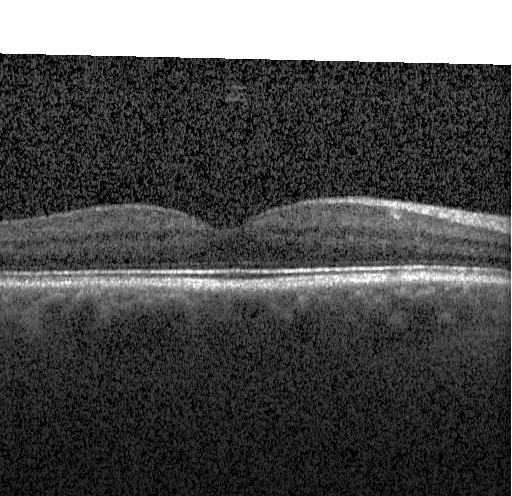 Impression: no evidence of choroidal neovascularization, diabetic macular edema, or drusen.